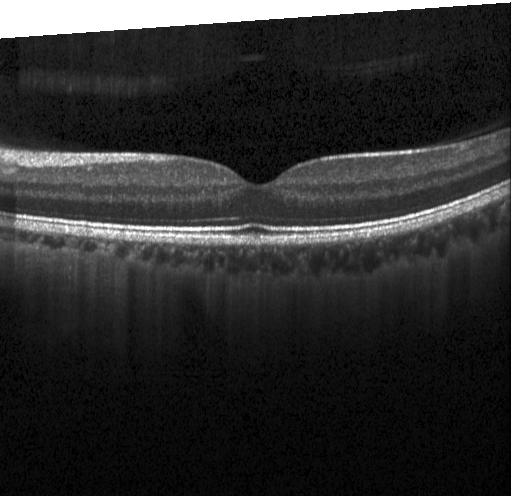
Impression: no evidence of choroidal neovascularization, diabetic macular edema, or drusen.